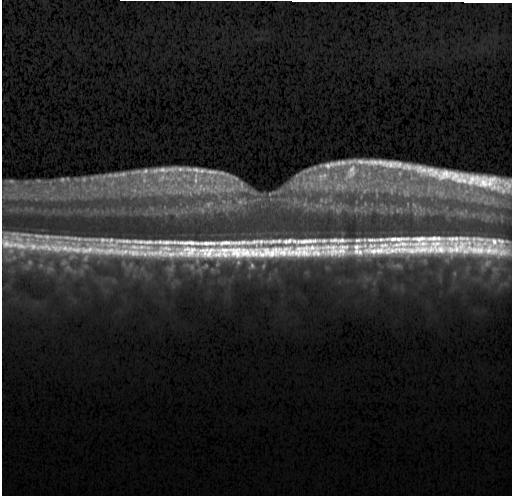

OCT B-scan; spectral-domain optical coherence tomography.
Finding: no choroidal neovascularization, no diabetic macular edema, and no drusen.